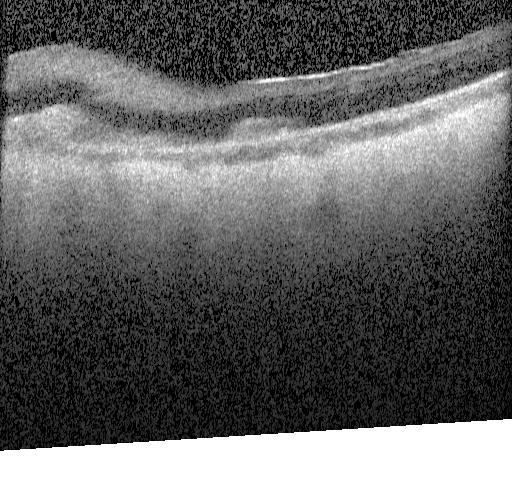

Fovea-centered; retinal OCT cross-section; Heidelberg Spectralis; SD-OCT.
Diagnosis: a choroidal neovascular membrane.